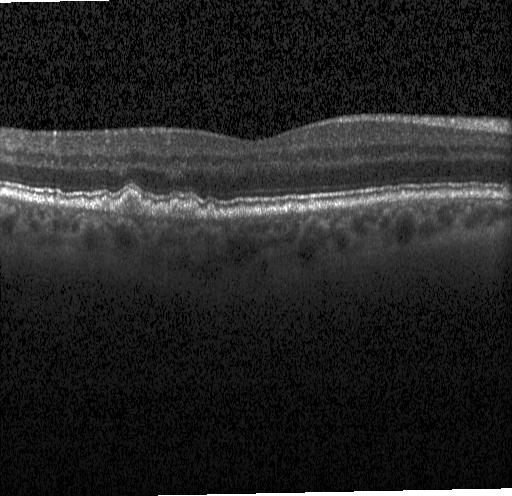 Heidelberg Spectralis; centered on the fovea; OCT B-scan.
Sub-RPE drusenoid deposits.